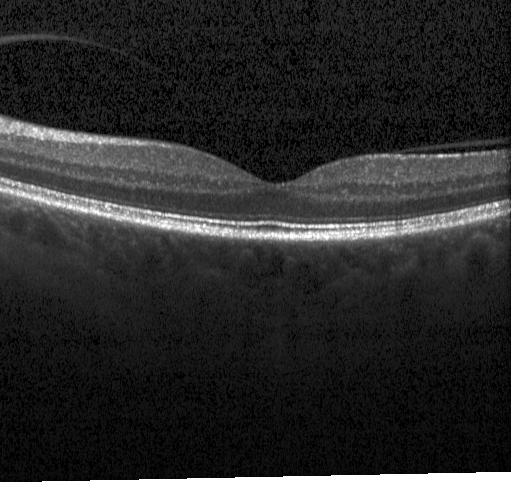

Optical coherence tomography scan · through the macula — The scan shows no CNV, no DME, and no drusen.